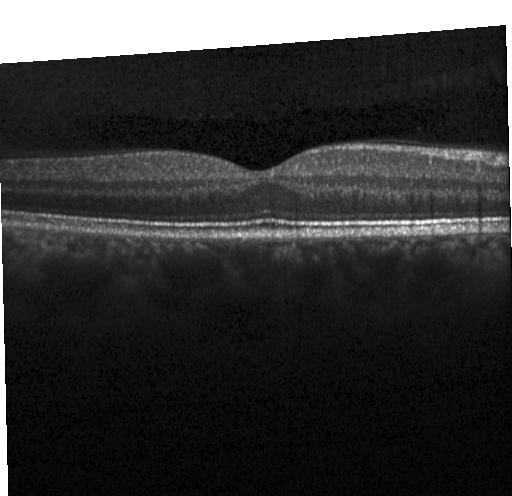

Diagnosis: no CNV, no DME, and no drusen.